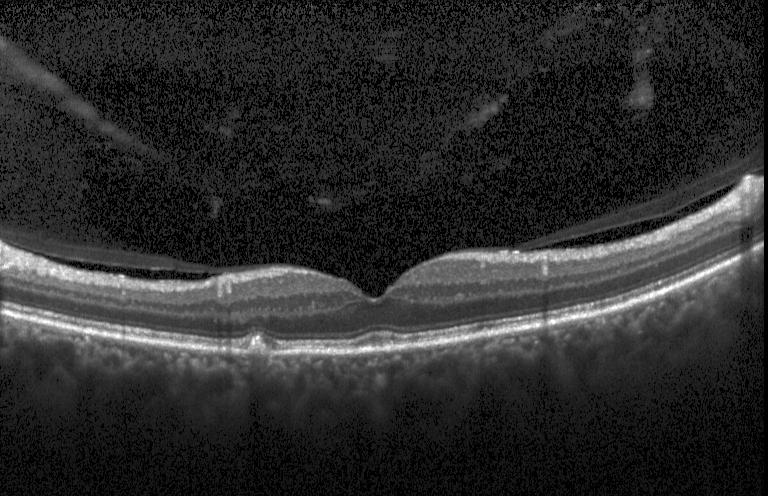
Diagnosis: drusen.